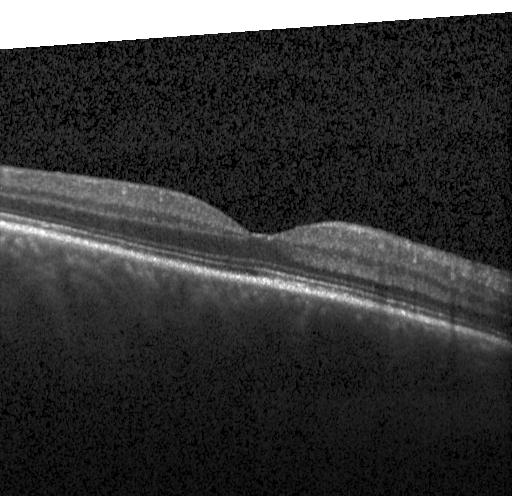

Diagnosis: no evidence of choroidal neovascularization, diabetic macular edema, or drusen.